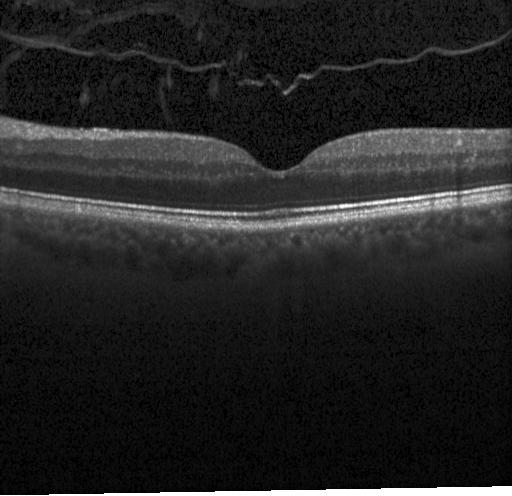 Optical coherence tomography scan.
Impression: neither choroidal neovascularization, diabetic macular edema, nor drusen.